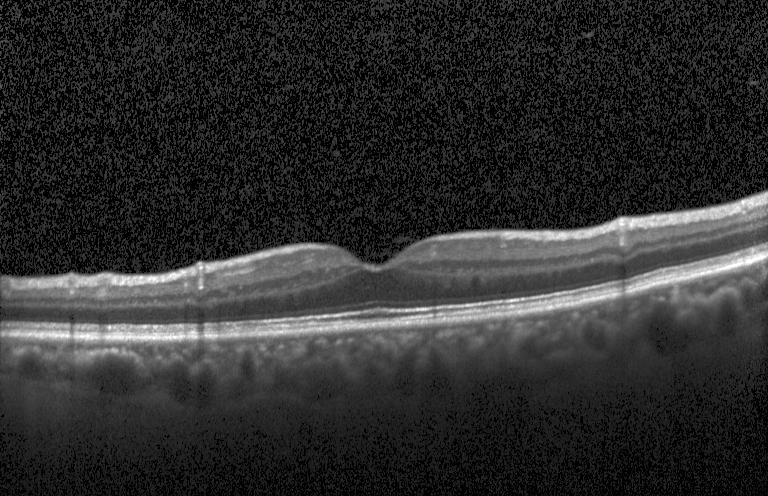
Centered on the fovea. OCT line scan. This B-scan demonstrates no evidence of CNV, DME, or drusen.